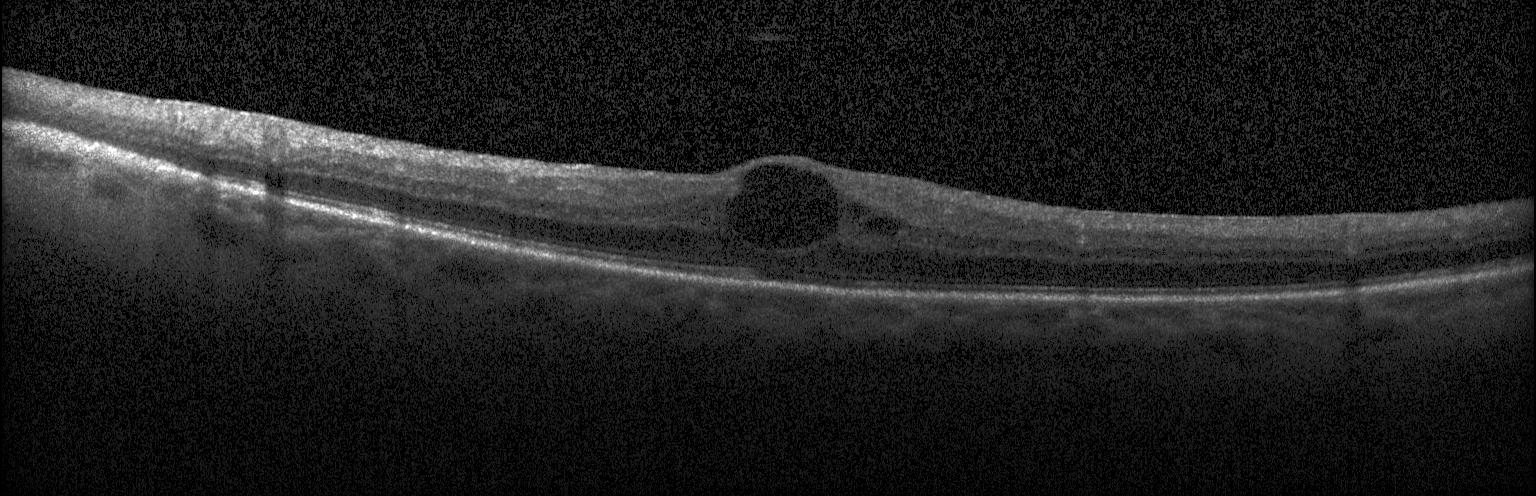

Optical coherence tomography scan. Finding: diabetic macular edema (DME).